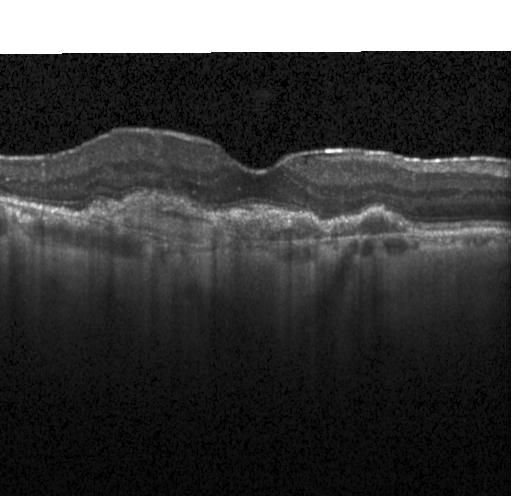

Spectral-domain optical coherence tomography · centered on the fovea · retinal OCT cross-section.
Diagnosis: CNV.